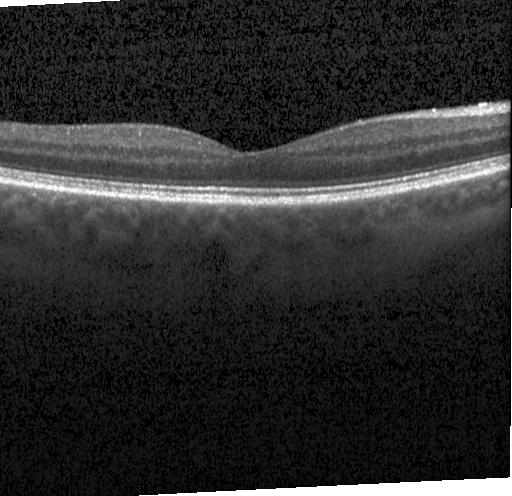

Horizontal scan through the fovea. SD-OCT. Optical coherence tomography B-scan. Instrument: Heidelberg Spectralis — The scan shows no CNV, DME, or drusen.